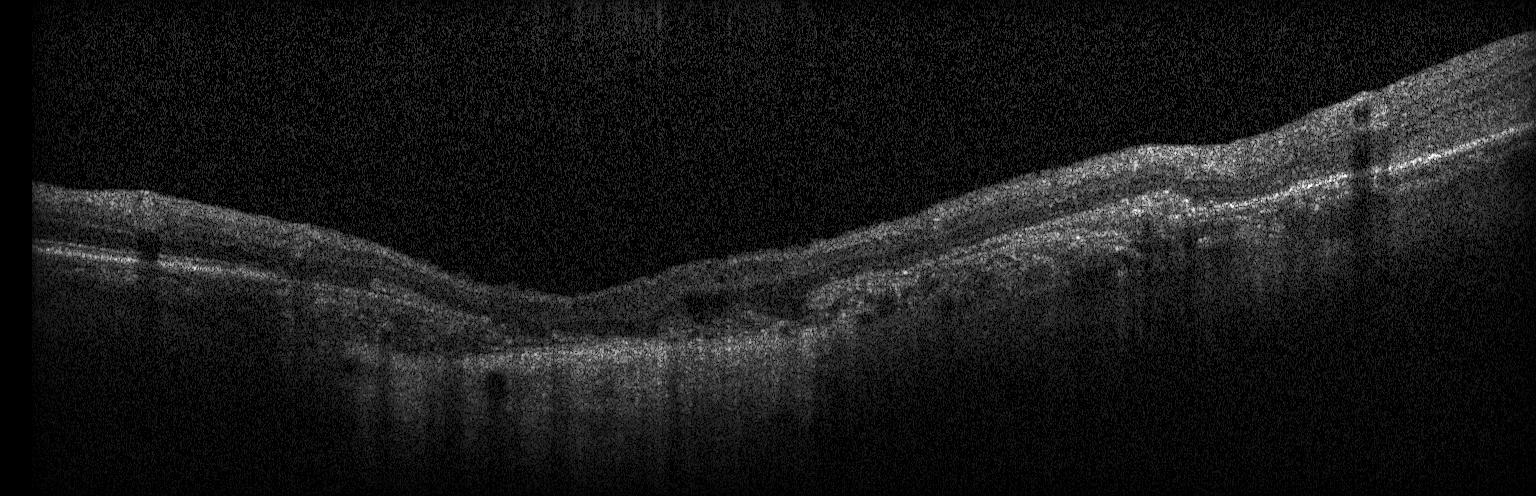

Optical coherence tomography scan. Heidelberg Spectralis.
Finding: choroidal neovascularization.